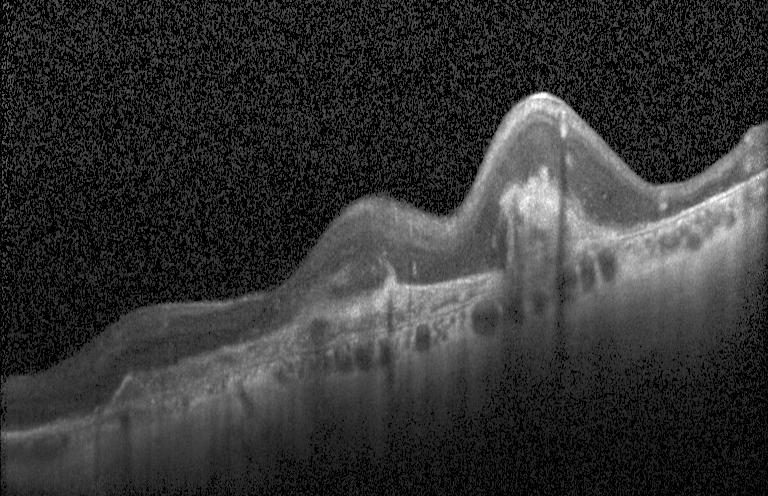

Diagnosis: CNV.